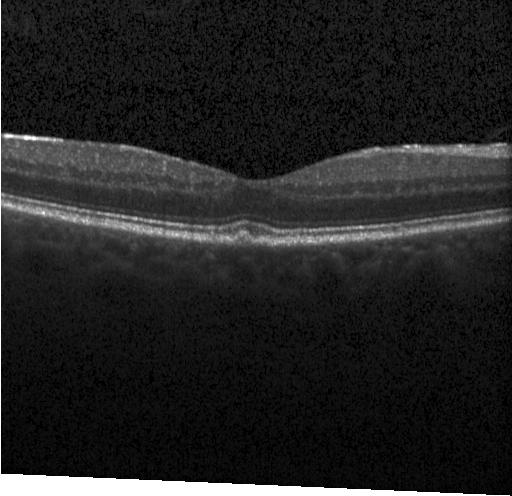

Diagnosis: drusen.